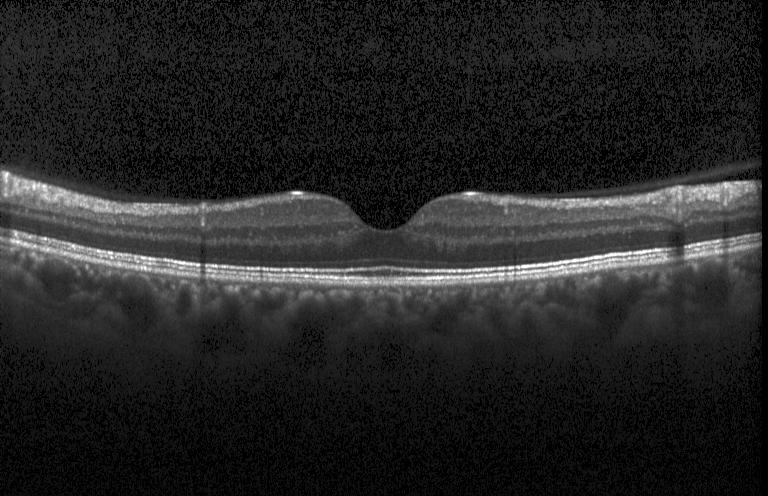
Fovea-centered, retinal OCT B-scan
Assessment: no choroidal neovascularization, no diabetic macular edema, and no drusen.